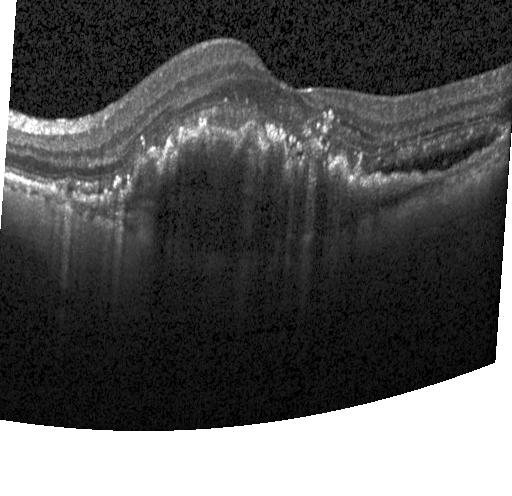 Heidelberg Spectralis OCT system. OCT B-scan.
The scan shows CNV.